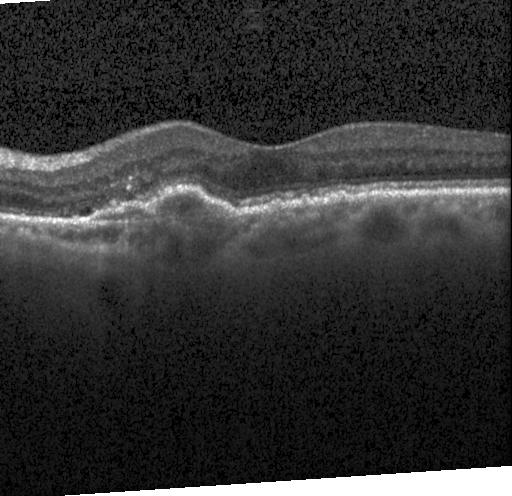

SD-OCT, retinal OCT cross-section — Diagnosis: a choroidal neovascular membrane.